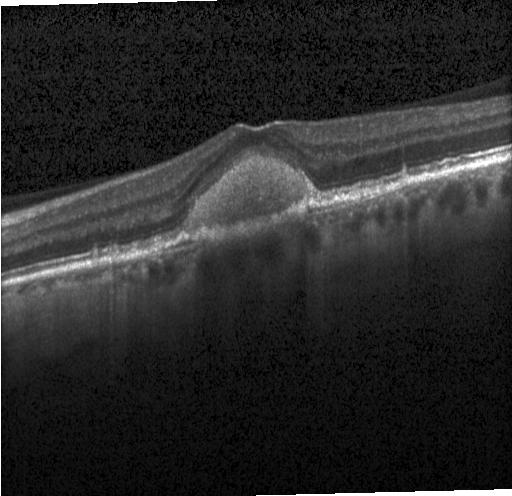
Finding: CNV.